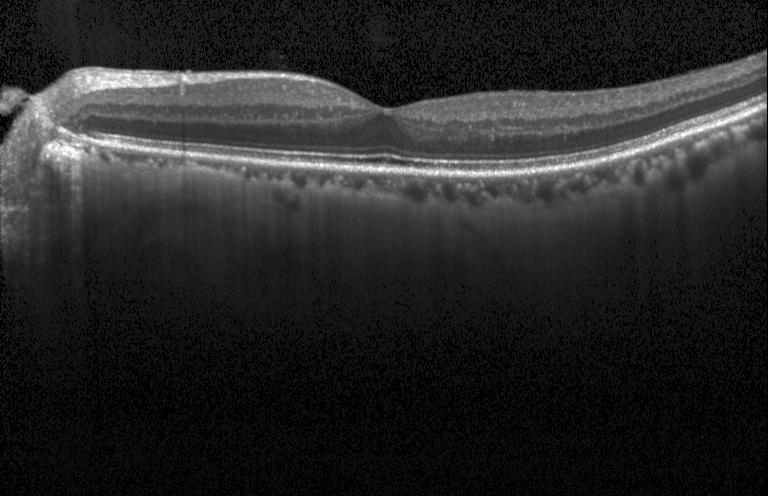
Horizontal scan through the fovea. Optical coherence tomography B-scan. Dx: no choroidal neovascularization, diabetic macular edema, or drusen.